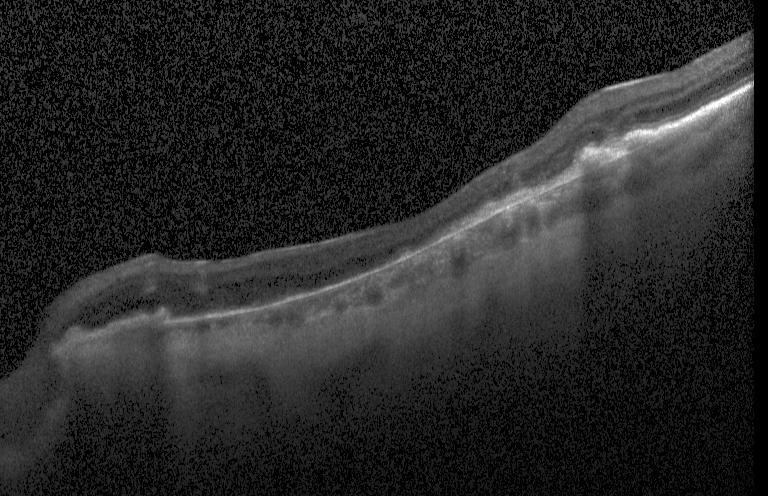 Instrument: Heidelberg Spectralis; spectral-domain optical coherence tomography; retinal OCT cross-section — Diagnosis: a choroidal neovascular membrane.